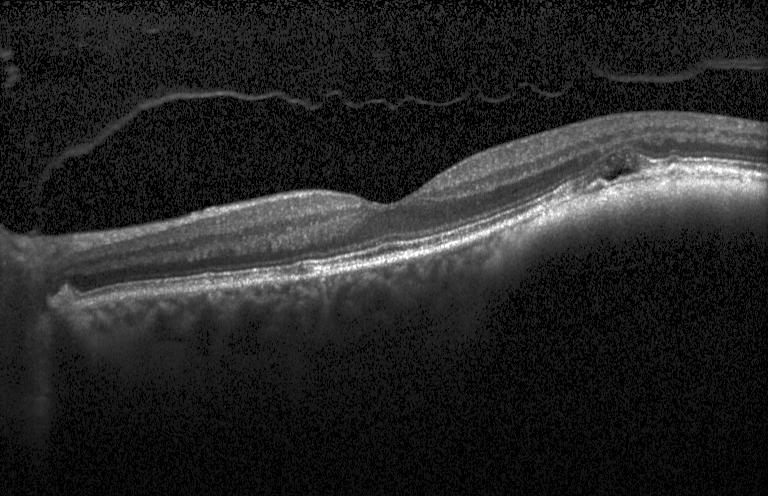

Macular OCT: choroidal neovascularization (CNV).